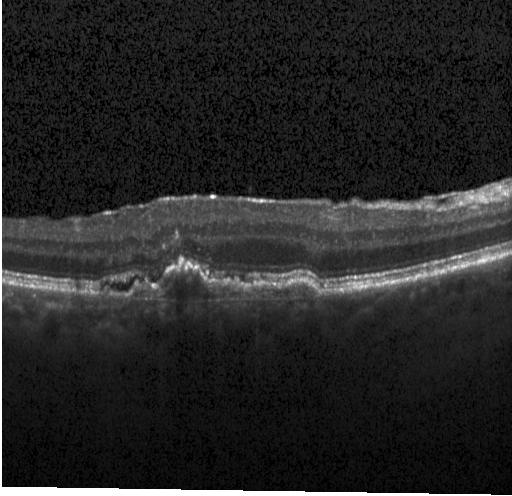

Retinal OCT cross-section showing a choroidal neovascular membrane.